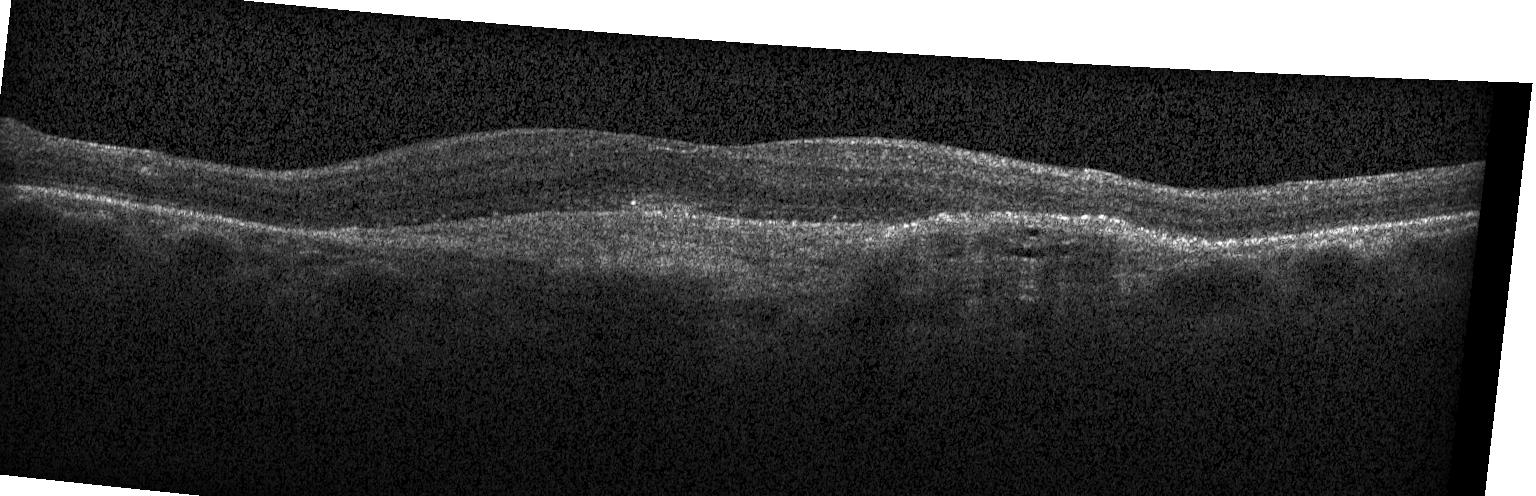 The scan shows a choroidal neovascular membrane.